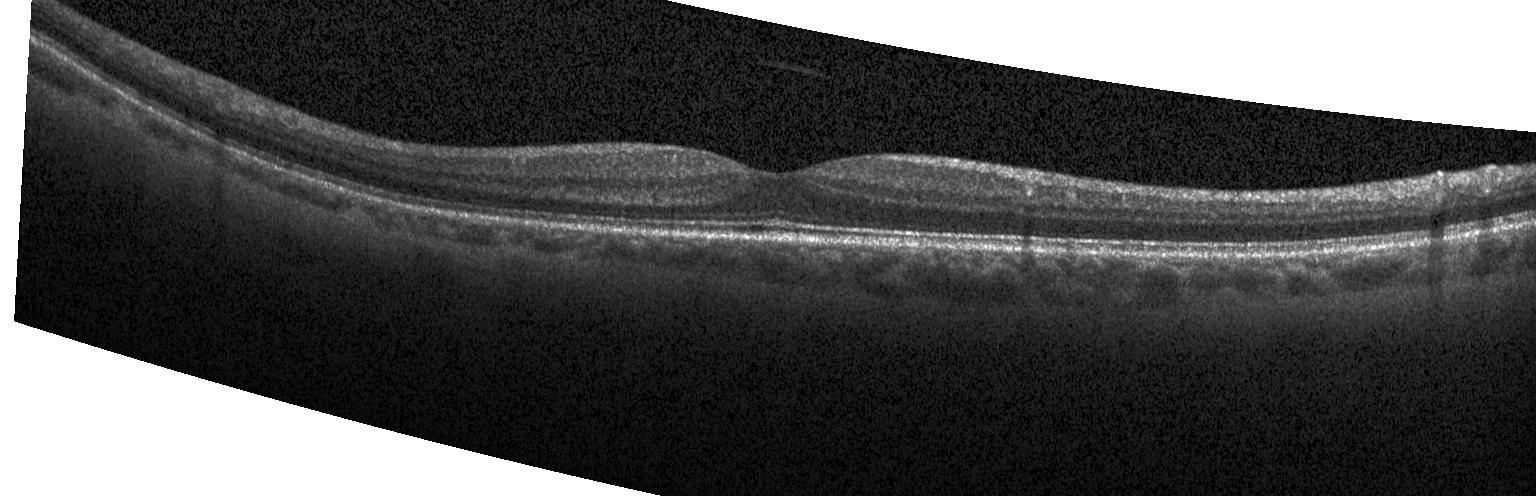 Heidelberg Spectralis OCT system. OCT B-scan. SD-OCT
The scan shows no evidence of CNV, DME, or drusen.